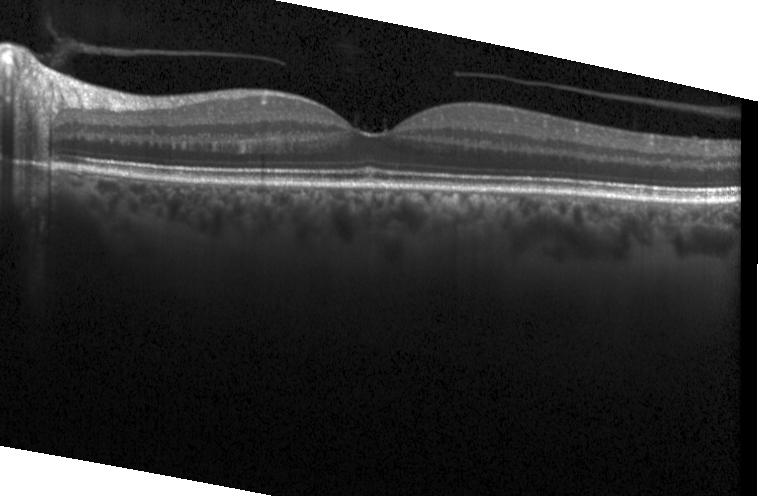 Impression: neither choroidal neovascularization, diabetic macular edema, nor drusen.